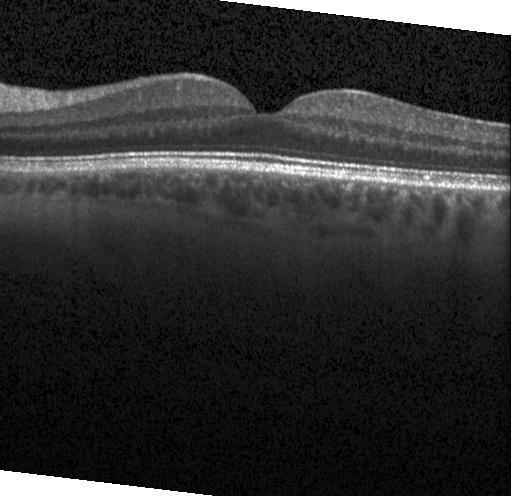 Spectral-domain optical coherence tomography. Through the macula. Acquired on a Heidelberg Spectralis. Retinal OCT B-scan
OCT finding: no evidence of CNV, DME, or drusen.